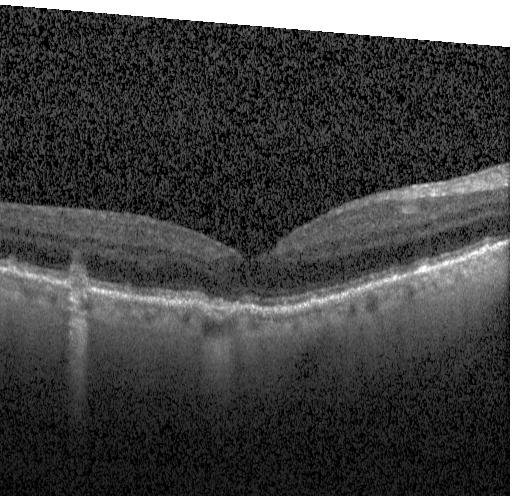
Optical coherence tomography scan, fovea-centered, SD-OCT, acquired on a Heidelberg Spectralis — Finding: drusen.